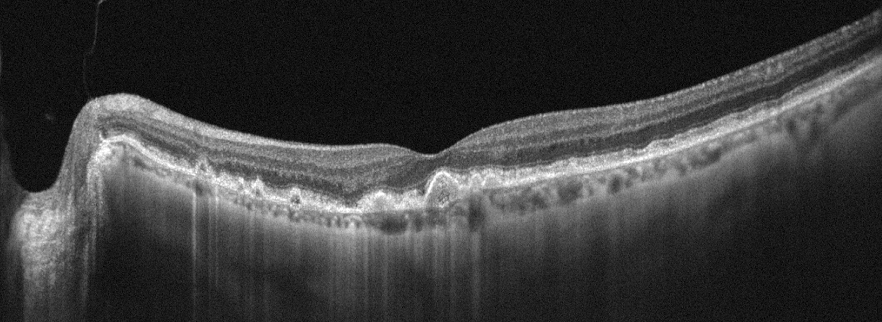 Optovue Avanti RTVue XR, OS, retinal OCT B-scan
Diagnosis: age-related macular degeneration (AMD).